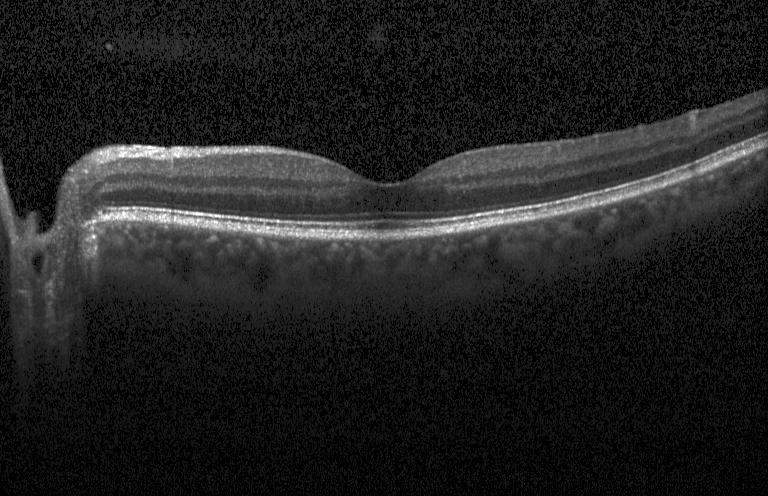
Macular OCT demonstrating neither CNV, DME, nor drusen.